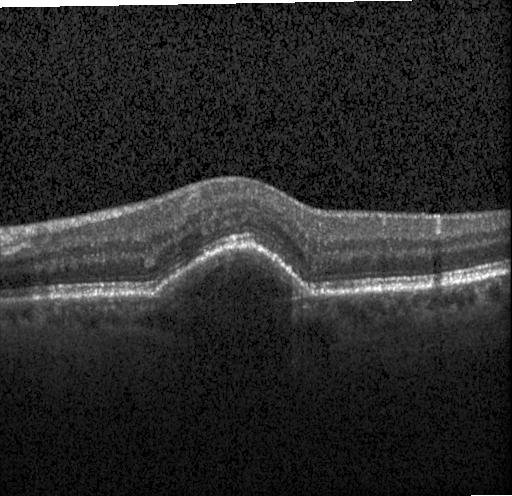 The scan shows choroidal neovascularization.